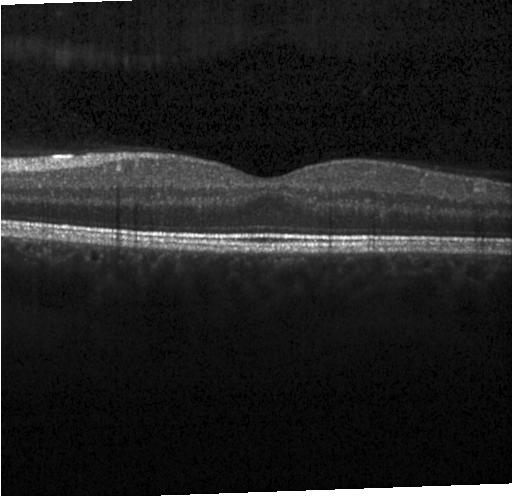

Retinal OCT cross-section showing neither CNV, DME, nor drusen.